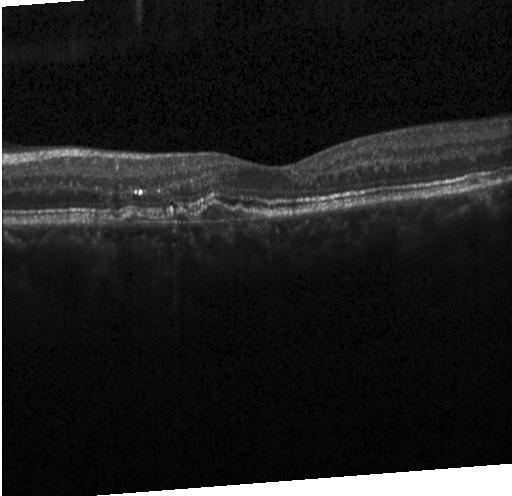

Spectral-domain OCT, Heidelberg Spectralis, retinal OCT B-scan.
Assessment: a choroidal neovascular membrane.